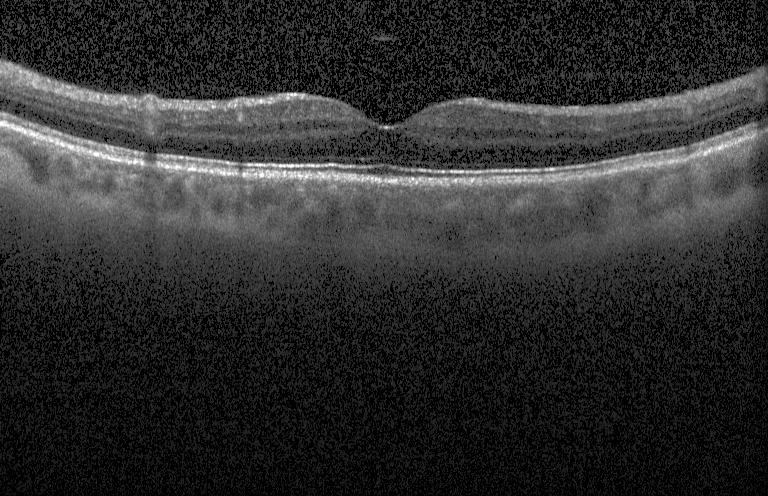 OCT scan showing no choroidal neovascularization, no diabetic macular edema, and no drusen.